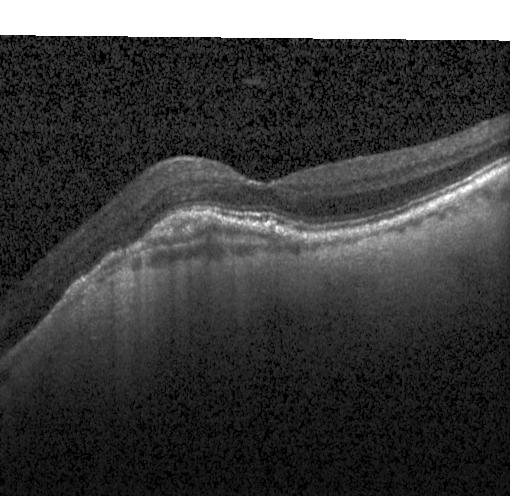 Horizontal scan through the fovea · OCT B-scan.
Choroidal neovascularization (CNV).